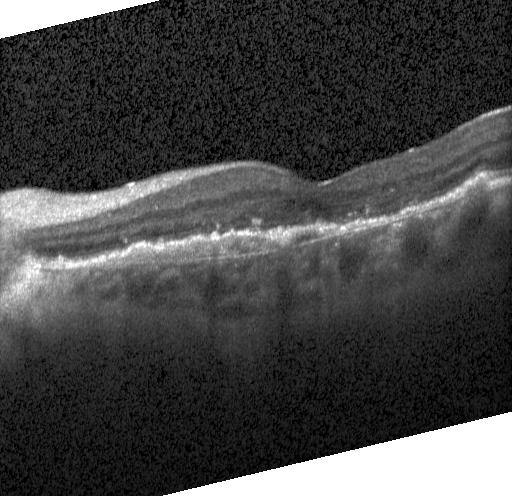 Retinal OCT B-scan · SD-OCT · Heidelberg Spectralis.
The scan shows choroidal neovascularization.